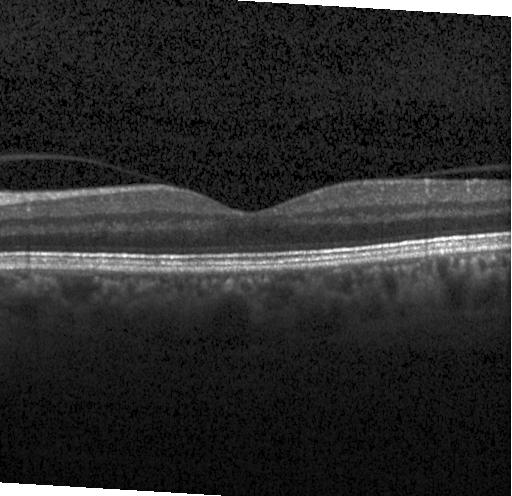

Instrument: Heidelberg Spectralis, optical coherence tomography B-scan, SD-OCT, centered on the fovea — The scan shows no evidence of choroidal neovascularization, diabetic macular edema, or drusen.